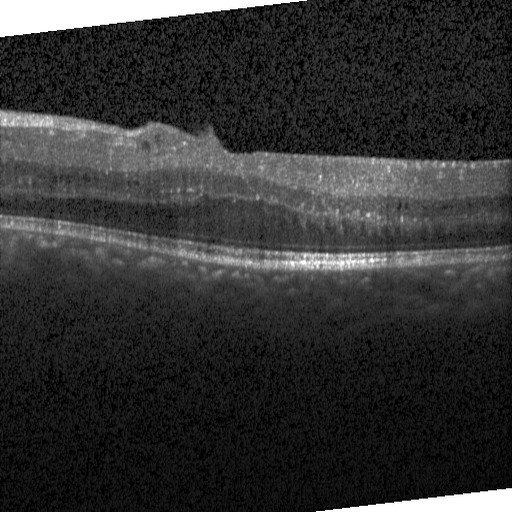 Impression: diabetic macular edema.